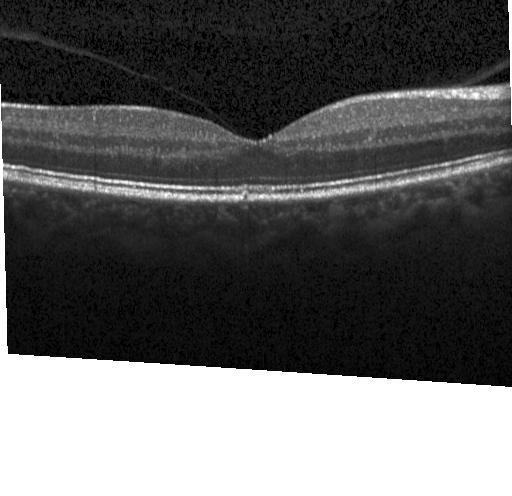 Impression: sub-RPE drusenoid deposits.